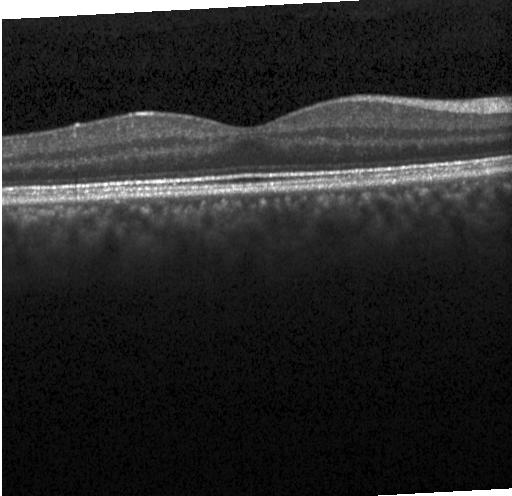
Assessment: no evidence of choroidal neovascularization, diabetic macular edema, or drusen.